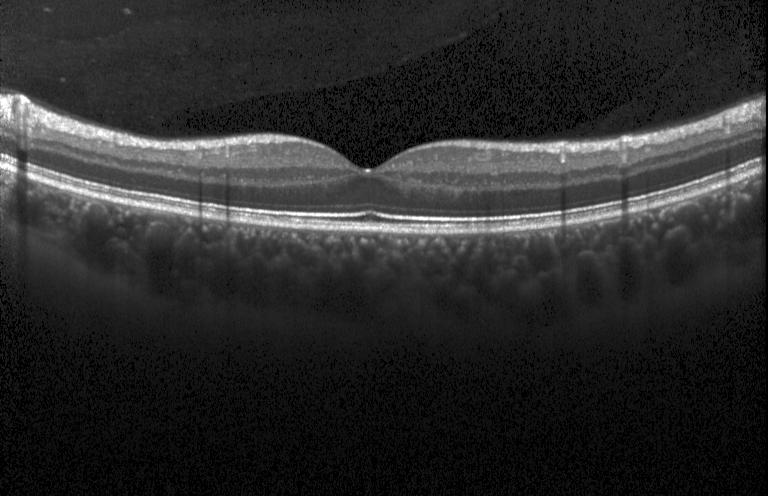

OCT B-scan
Dx: neither choroidal neovascularization, diabetic macular edema, nor drusen.